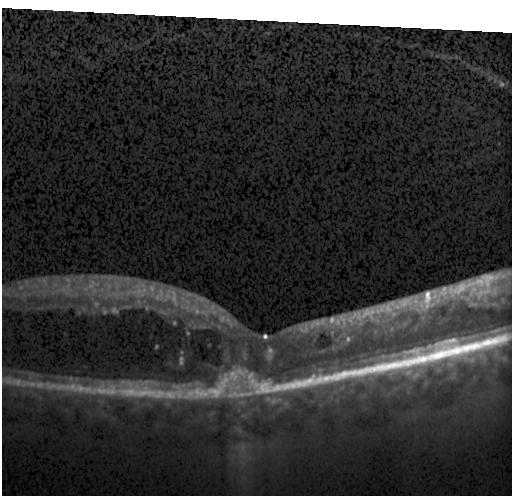
Heidelberg Spectralis · centered on the fovea · spectral-domain optical coherence tomography · optical coherence tomography B-scan. Dx: DME.